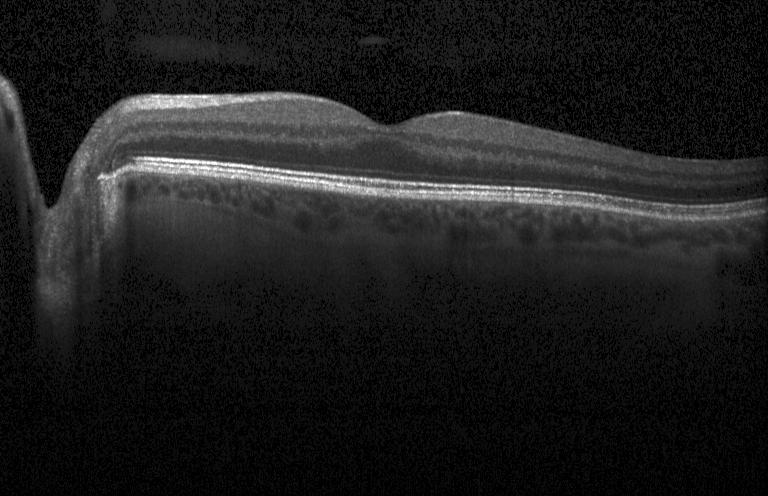
Retinal OCT cross-section · Heidelberg Spectralis OCT system.
No choroidal neovascularization, diabetic macular edema, or drusen.